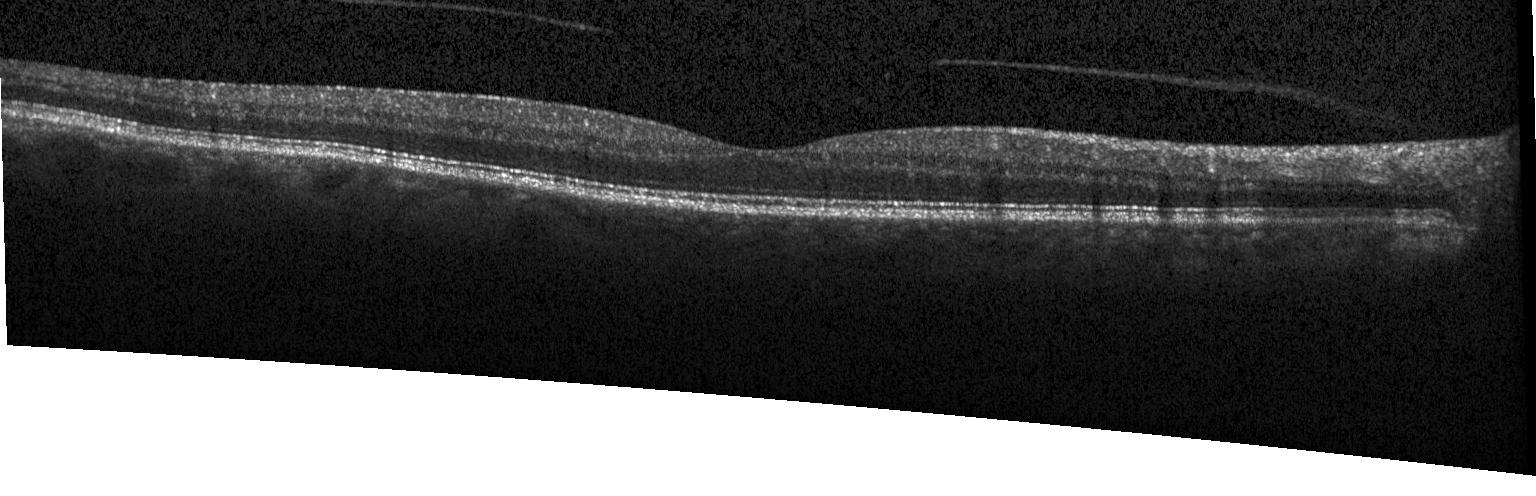
Spectral-domain optical coherence tomography; retinal OCT cross-section; Heidelberg Spectralis OCT system; horizontal scan through the fovea.
Dx: neither choroidal neovascularization, diabetic macular edema, nor drusen.